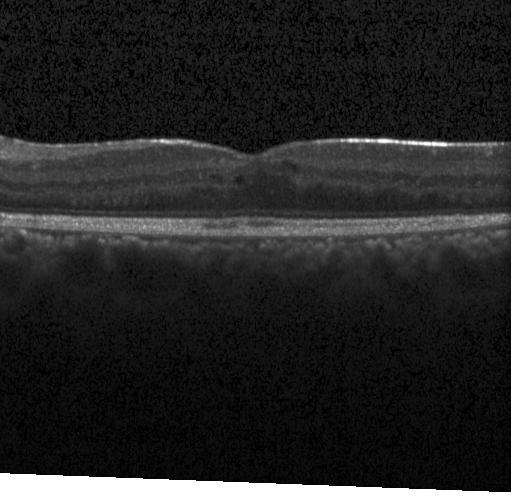
OCT scan showing diabetic macular edema.